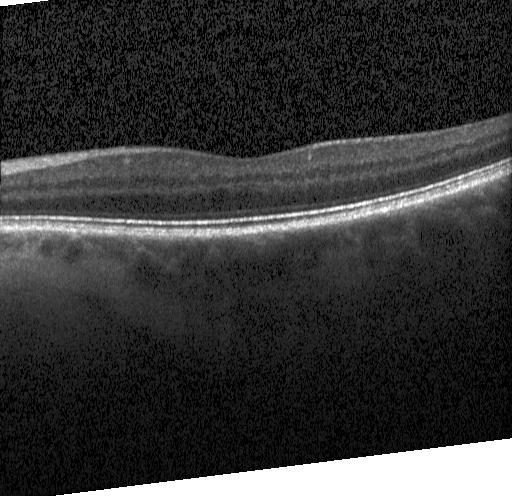

Optical coherence tomography scan · SD-OCT · centered on the fovea — Assessment: no CNV, DME, or drusen.